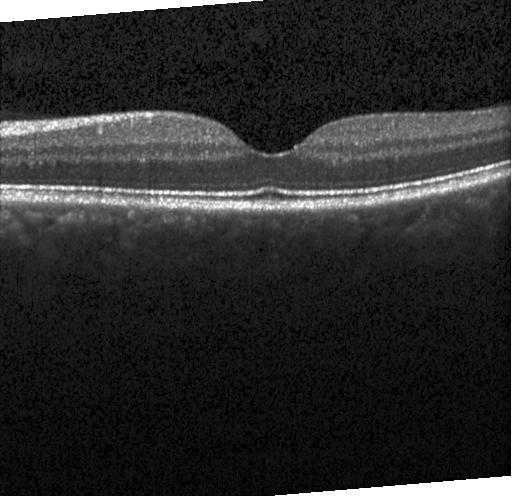
Retinal OCT cross-section showing no choroidal neovascularization, no diabetic macular edema, and no drusen.